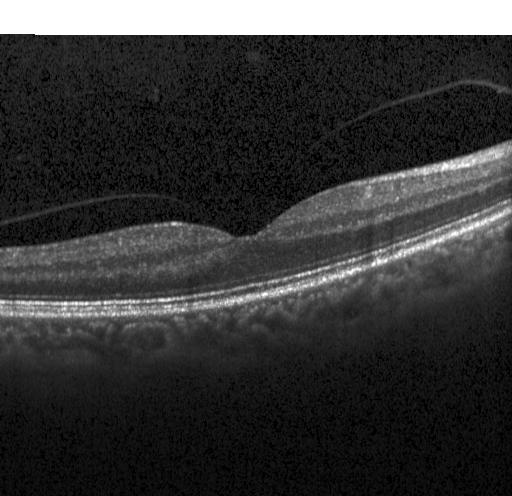 OCT B-scan, Heidelberg Spectralis OCT system.
Diagnosis: no choroidal neovascularization, no diabetic macular edema, and no drusen.